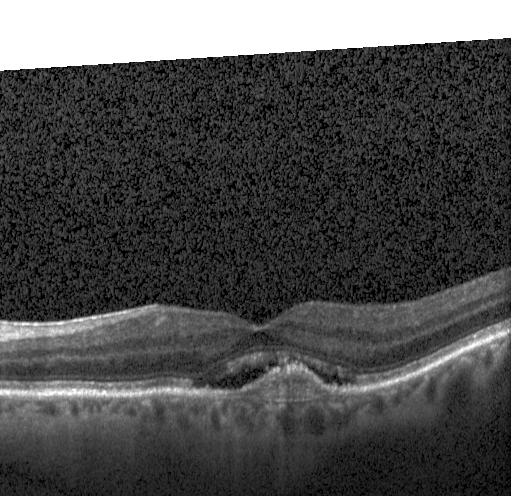

OCT B-scan. Assessment: choroidal neovascularization.